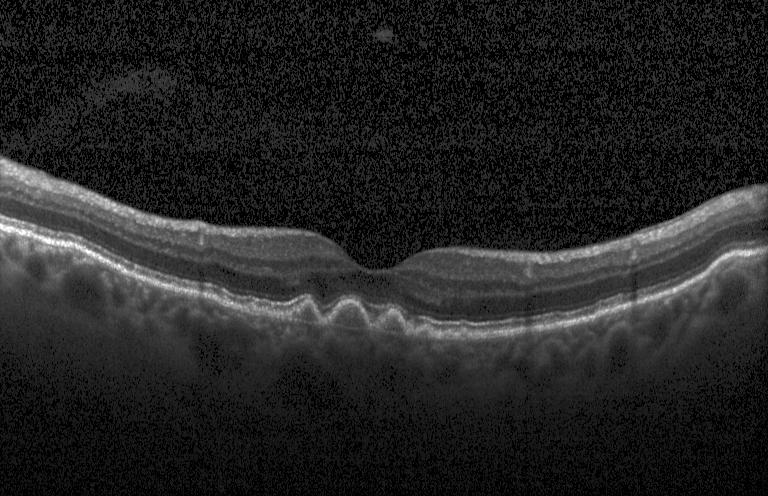

Instrument: Heidelberg Spectralis · optical coherence tomography B-scan · spectral-domain optical coherence tomography · centered on the fovea — Finding: drusen.